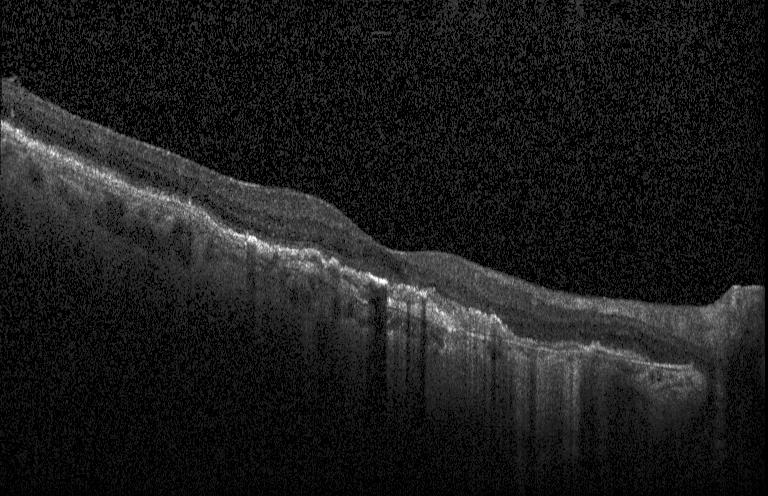
Instrument: Heidelberg Spectralis; optical coherence tomography scan; horizontal scan through the fovea; spectral-domain OCT
Macular OCT: a choroidal neovascular membrane.